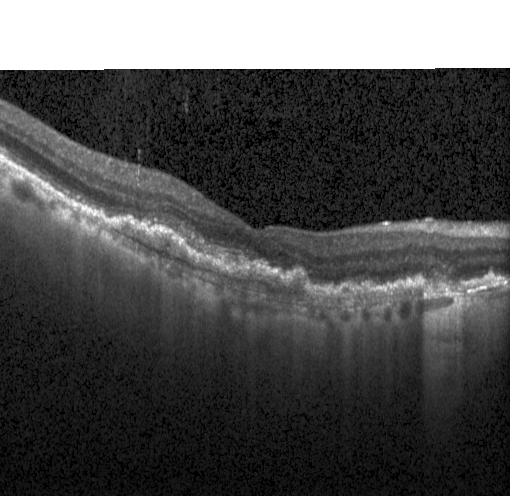 Impression: choroidal neovascularization.